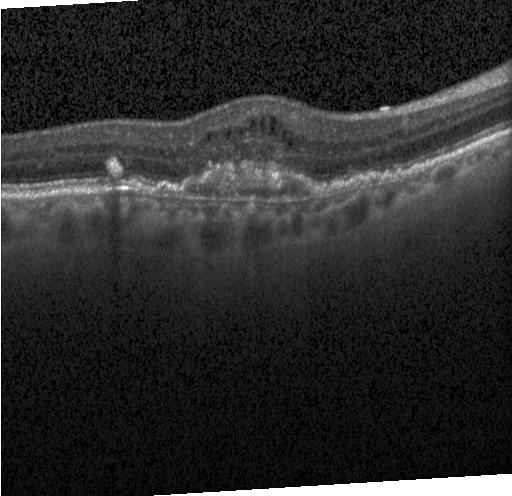

Retinal OCT cross-section; centered on the fovea; Heidelberg Spectralis OCT system; SD-OCT.
Impression: choroidal neovascularization.